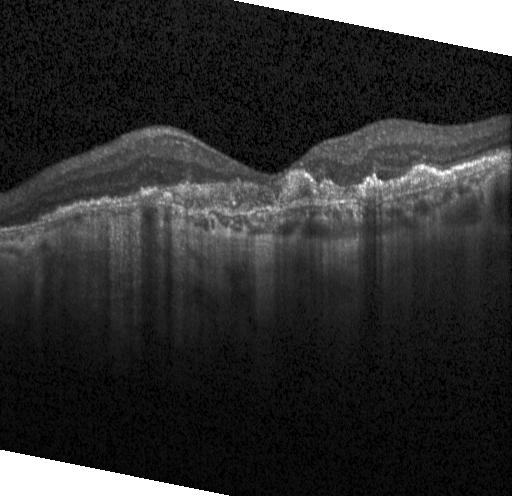
Macular OCT: a choroidal neovascular membrane.